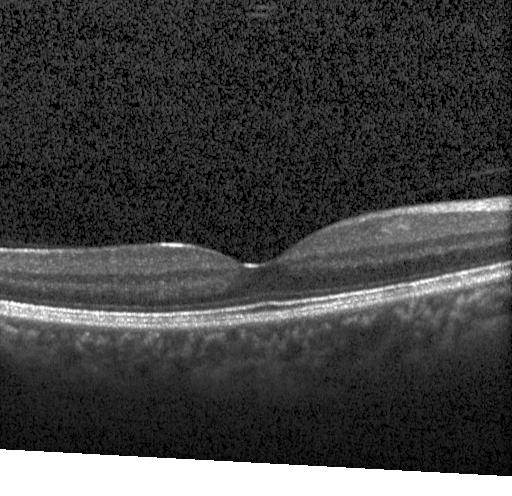 Macular OCT: no evidence of choroidal neovascularization, diabetic macular edema, or drusen.